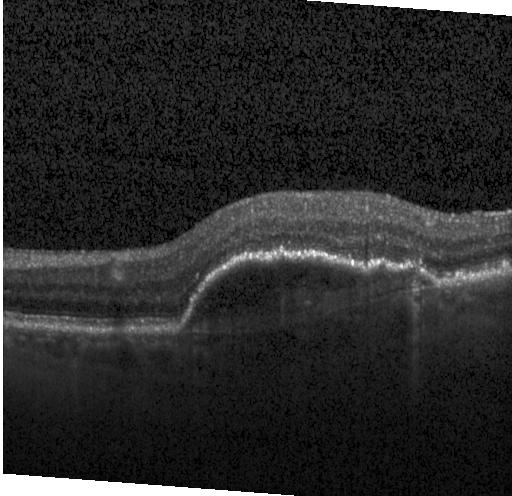 Acquired on a Heidelberg Spectralis; SD-OCT; OCT line scan; centered on the fovea.
Finding: a choroidal neovascular membrane.